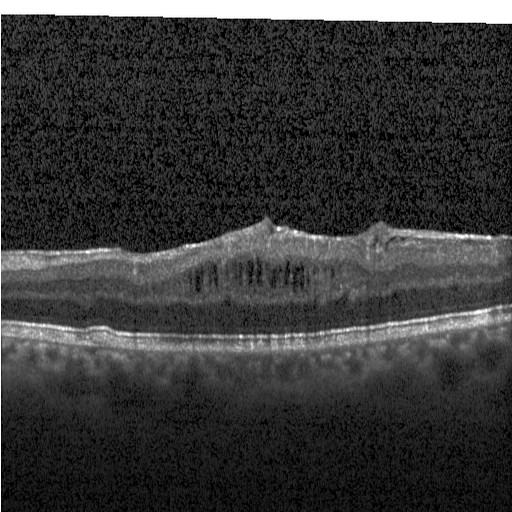

OCT finding: diabetic macular edema (DME).